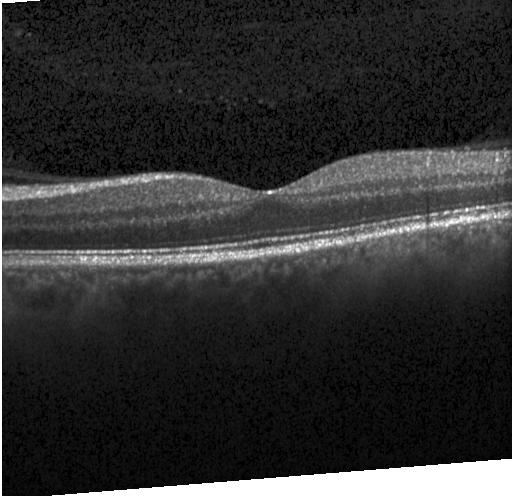 Macular scan. Optical coherence tomography B-scan.
No choroidal neovascularization, diabetic macular edema, or drusen.